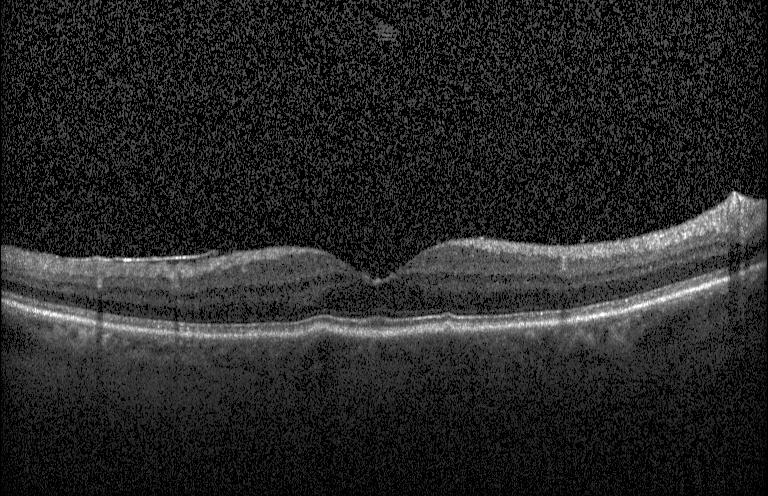 SD-OCT, OCT line scan, centered on the fovea
Impression: multiple drusen.